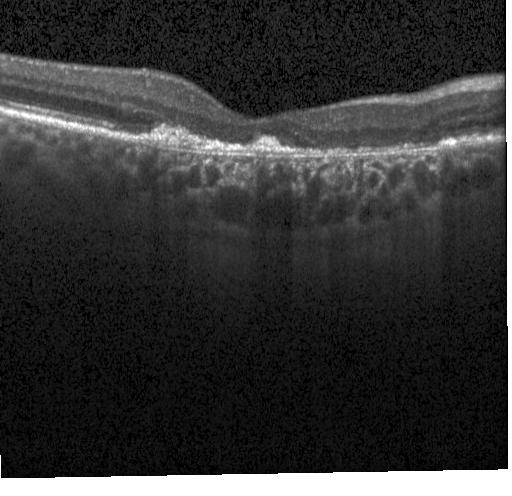
OCT line scan. Diagnosis: a choroidal neovascular membrane.